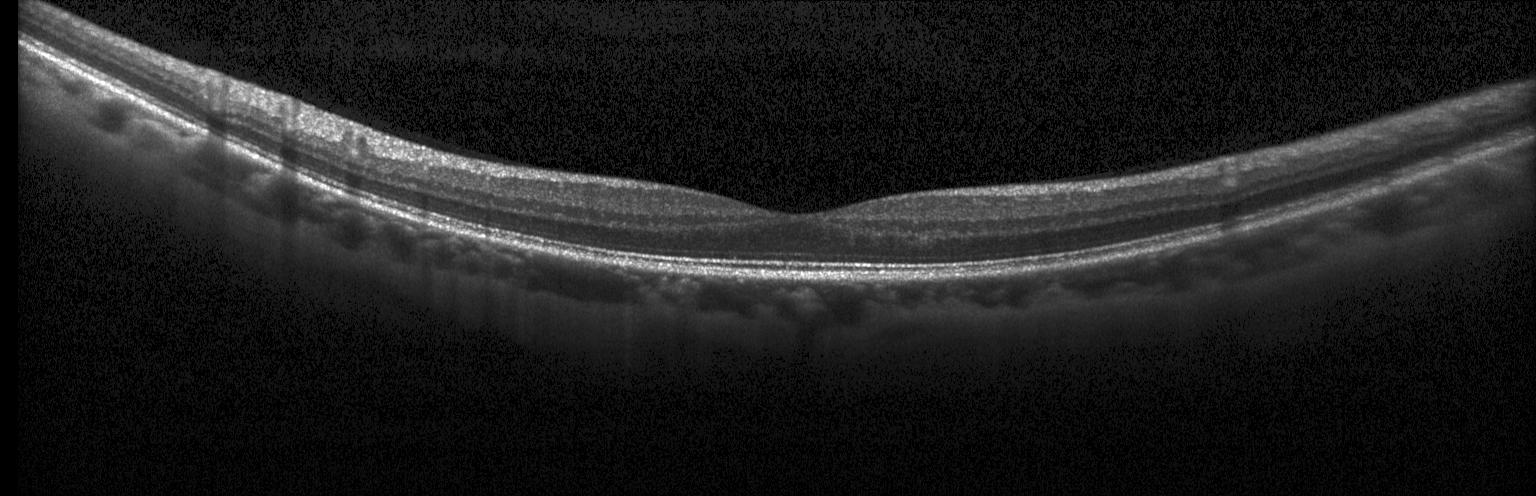
OCT line scan
Impression: neither CNV, DME, nor drusen.